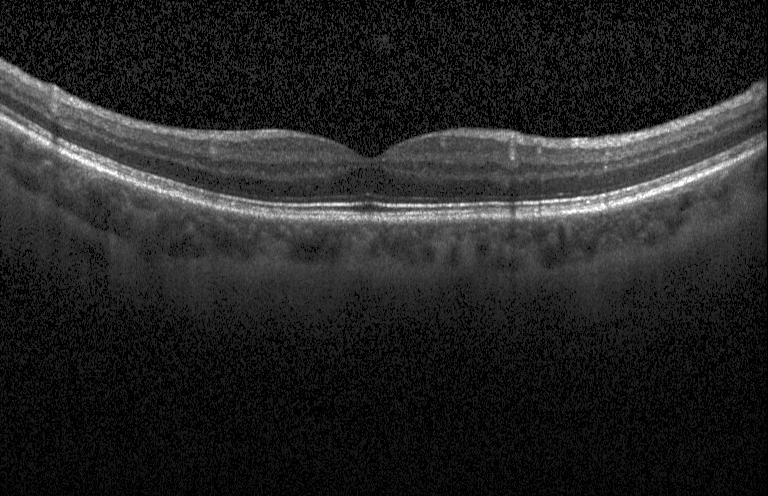

No choroidal neovascularization, diabetic macular edema, or drusen.